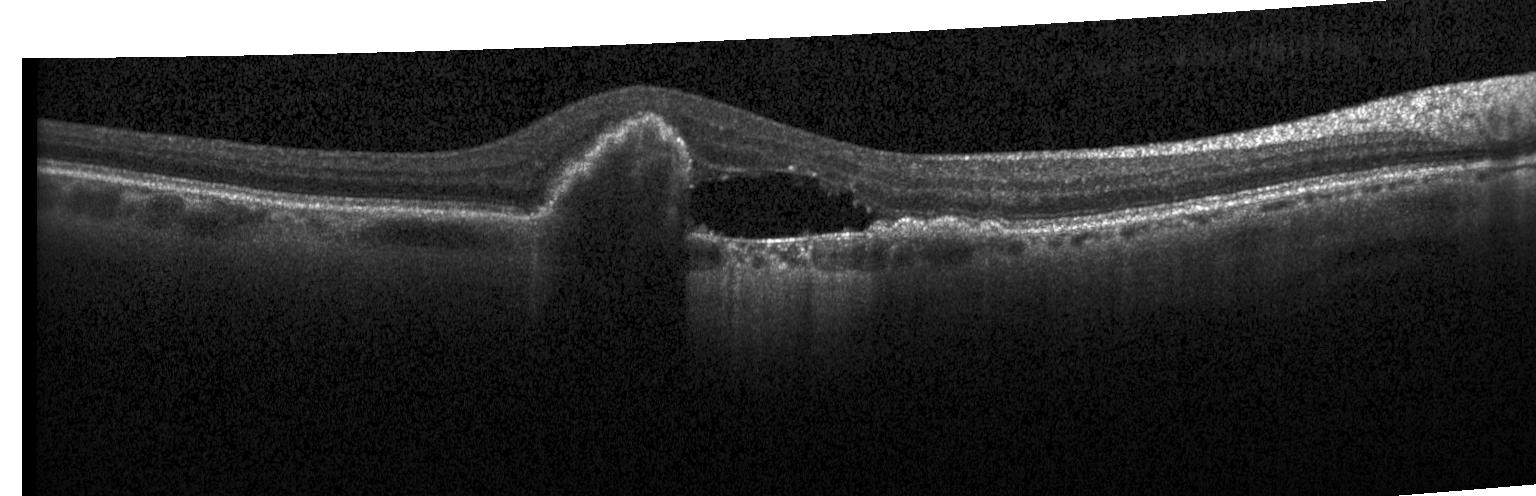
OCT B-scan, SD-OCT, fovea-centered.
Diagnosis: a choroidal neovascular membrane.